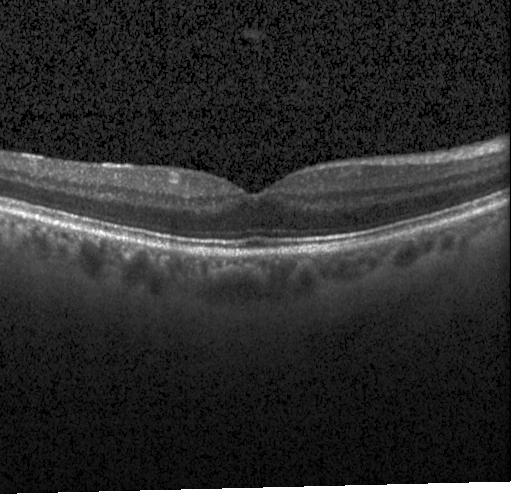

Optical coherence tomography scan; horizontal scan through the fovea
OCT finding: no CNV, no DME, and no drusen.